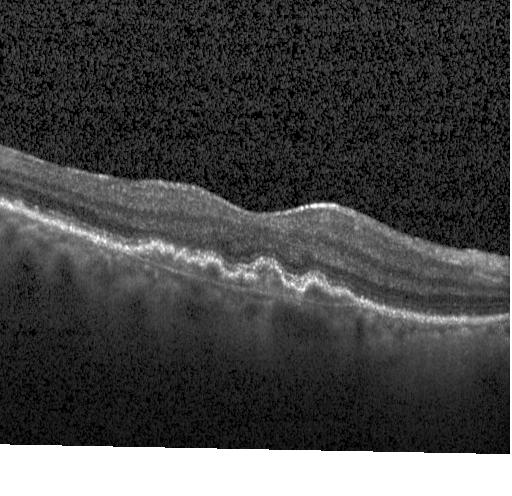
OCT finding: a choroidal neovascular membrane.